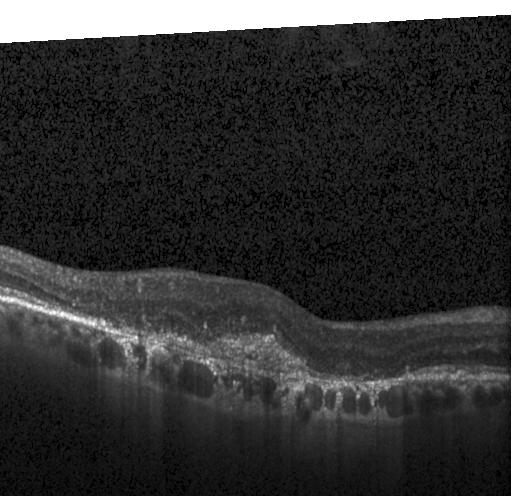
Through the macula, retinal OCT cross-section. OCT finding: choroidal neovascularization.